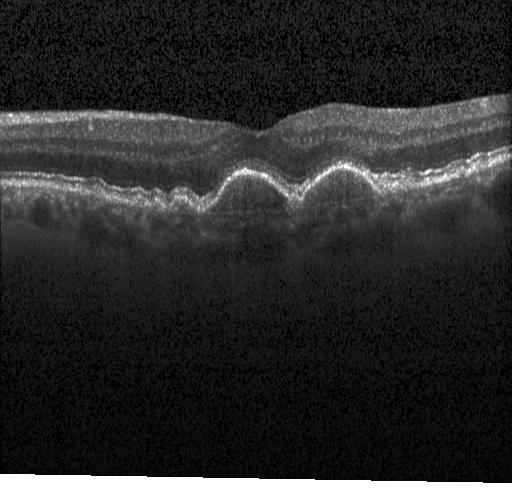
Centered on the fovea. Optical coherence tomography B-scan. Heidelberg Spectralis. This B-scan demonstrates drusen.